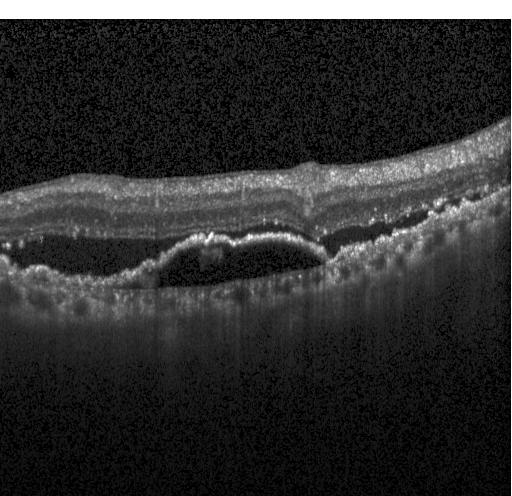

OCT B-scan · spectral-domain optical coherence tomography — Finding: a choroidal neovascular membrane.